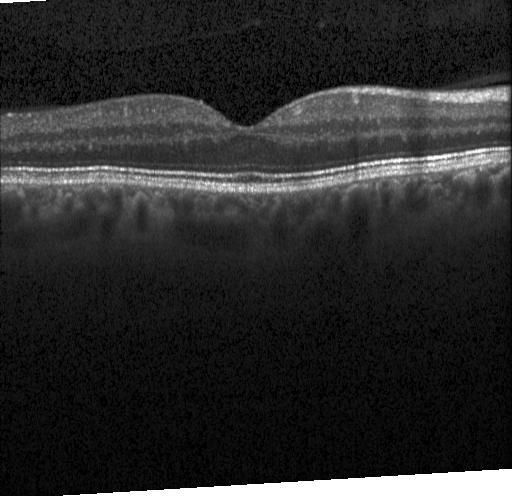 Spectral-domain optical coherence tomography · centered on the fovea · optical coherence tomography scan — Dx: no evidence of choroidal neovascularization, diabetic macular edema, or drusen.